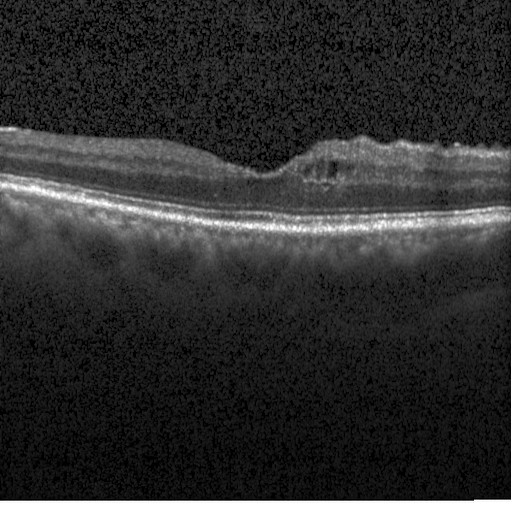 Optical coherence tomography scan
The scan shows DME.